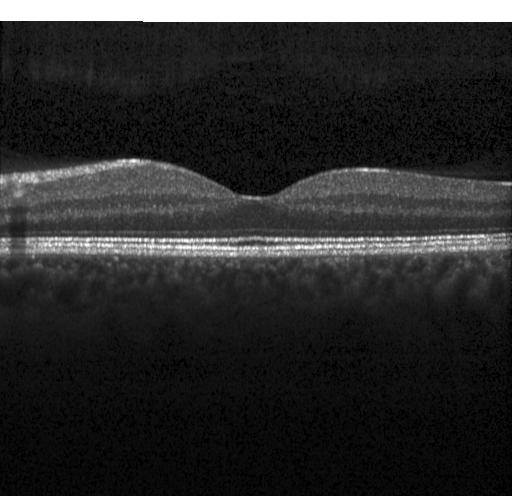

Retinal OCT cross-section · macular scan.
Finding: neither CNV, DME, nor drusen.